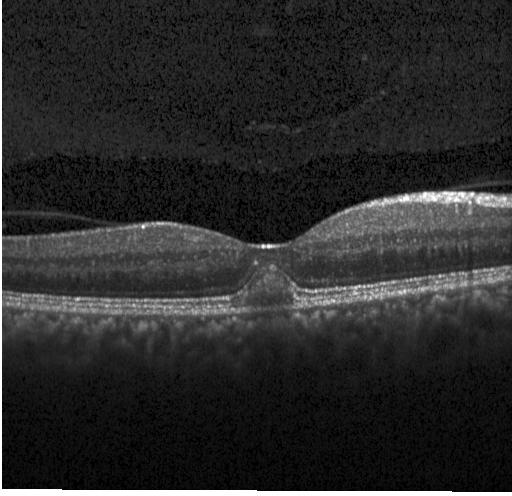 Diagnosis: a choroidal neovascular membrane.